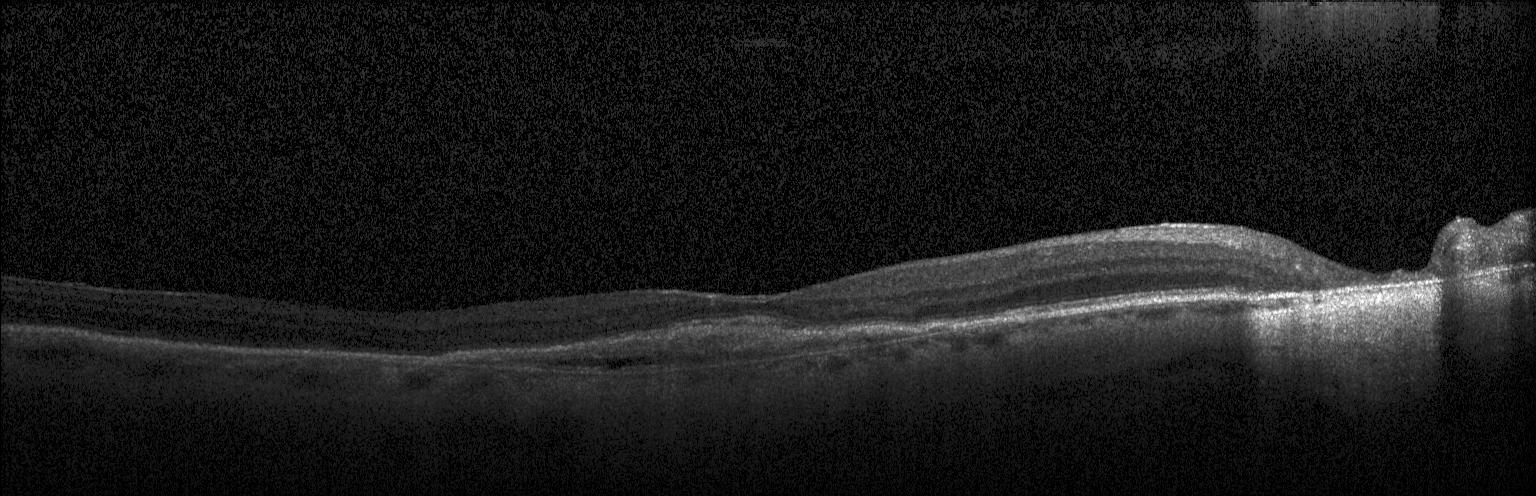

Diagnosis: choroidal neovascularization (CNV).